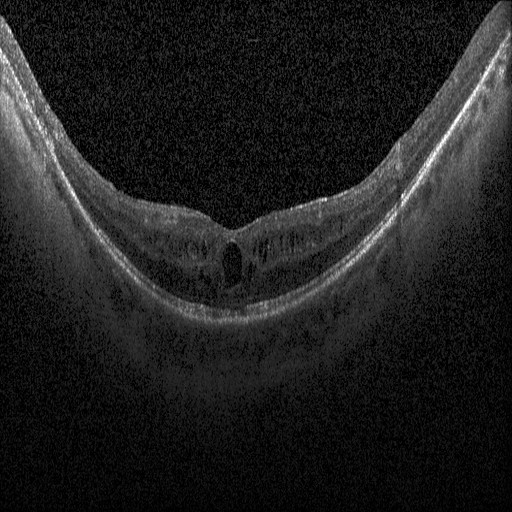 OCT scan showing DME.